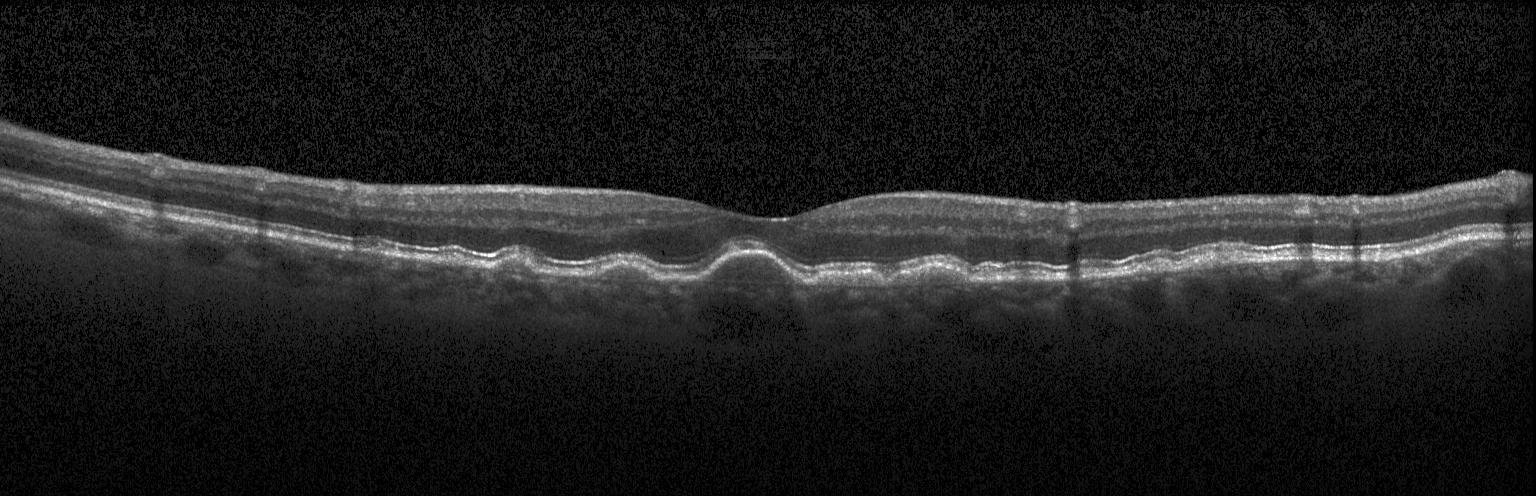
Assessment: sub-RPE drusenoid deposits.